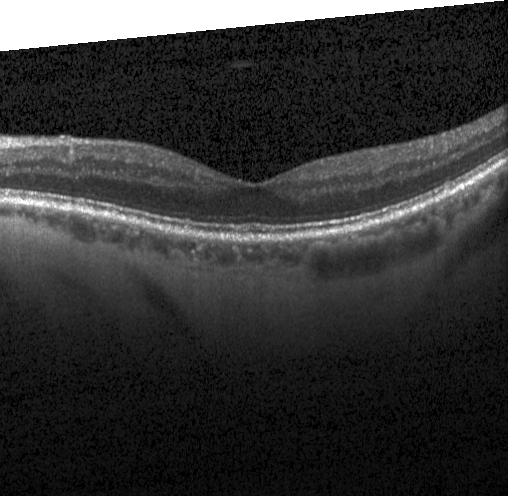

SD-OCT. OCT B-scan
Diagnosis: no CNV, no DME, and no drusen.